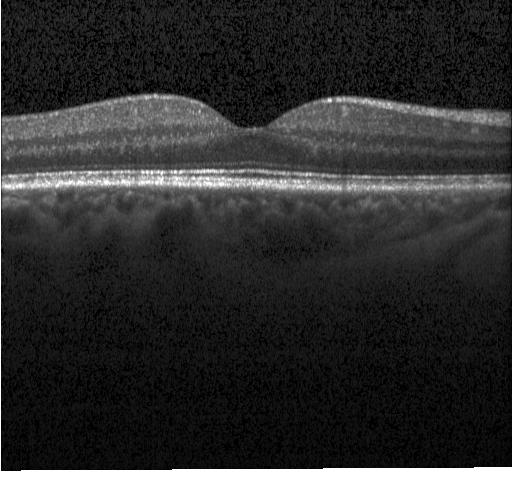 Centered on the fovea · OCT B-scan · acquired on a Heidelberg Spectralis
Assessment: no CNV, no DME, and no drusen.